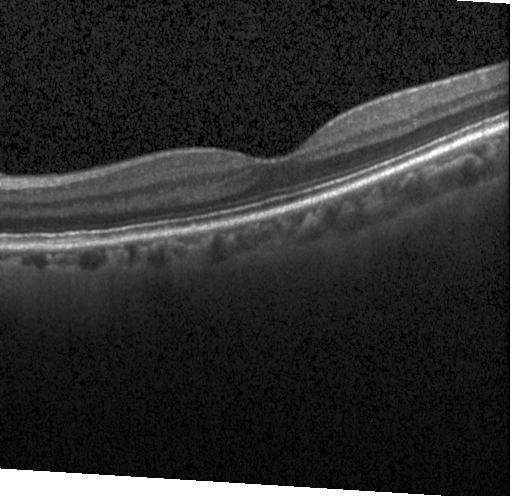

Diagnosis: no choroidal neovascularization, no diabetic macular edema, and no drusen.